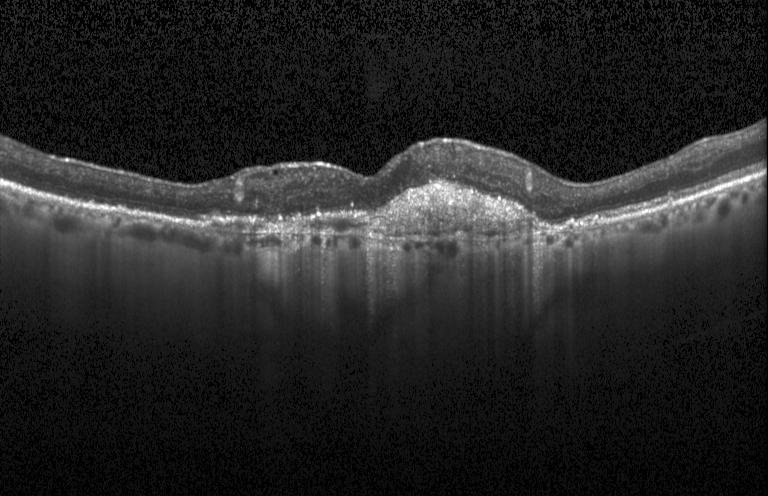

OCT scan showing a choroidal neovascular membrane.